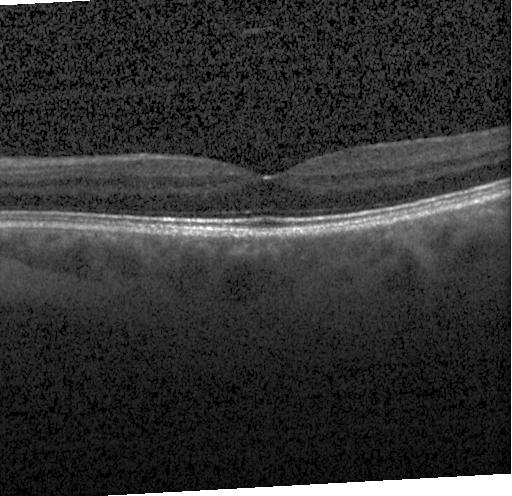 Optical coherence tomography B-scan.
Finding: no evidence of CNV, DME, or drusen.